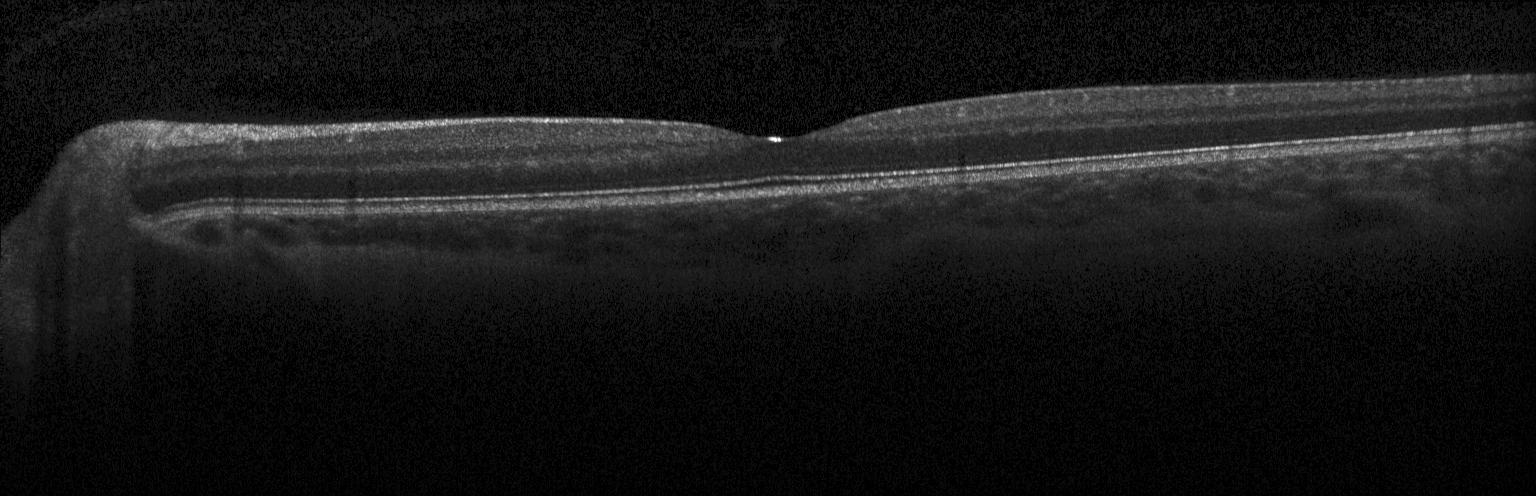
Macular OCT demonstrating neither choroidal neovascularization, diabetic macular edema, nor drusen.